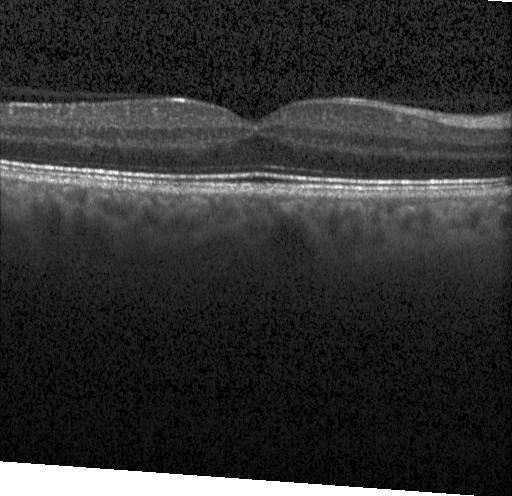
Fovea-centered, optical coherence tomography scan, Heidelberg Spectralis, spectral-domain OCT.
This B-scan demonstrates neither CNV, DME, nor drusen.